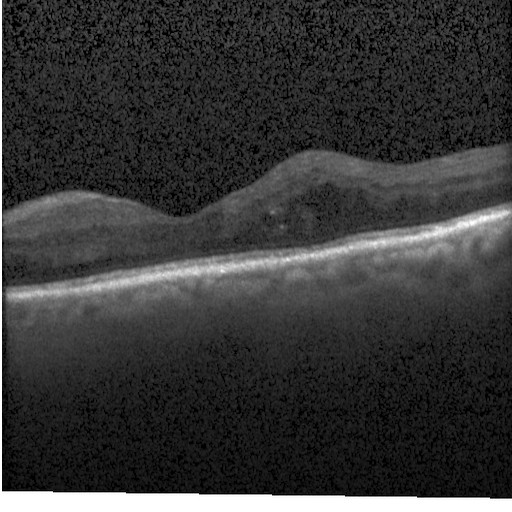

Optical coherence tomography B-scan. OCT finding: diabetic macular edema.